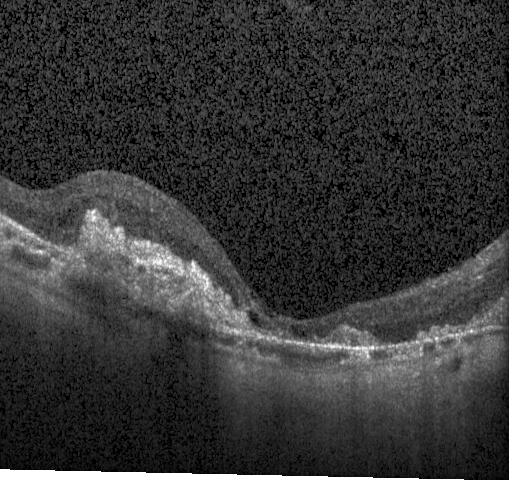 Horizontal scan through the fovea; optical coherence tomography scan; spectral-domain OCT. Diagnosis: choroidal neovascularization.